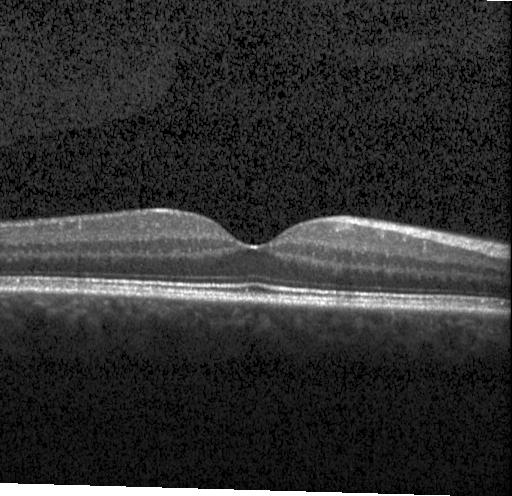

Finding: no evidence of choroidal neovascularization, diabetic macular edema, or drusen.